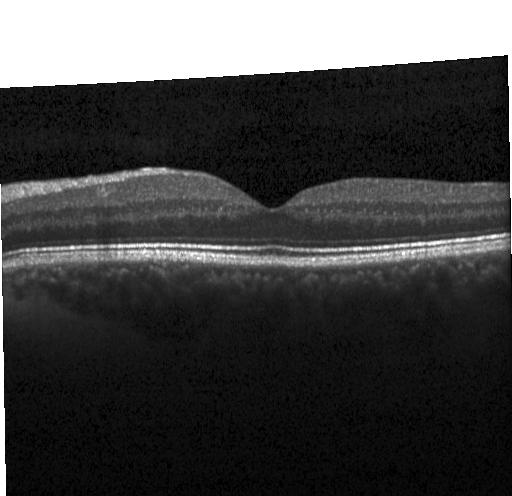
OCT B-scan. No choroidal neovascularization, no diabetic macular edema, and no drusen.